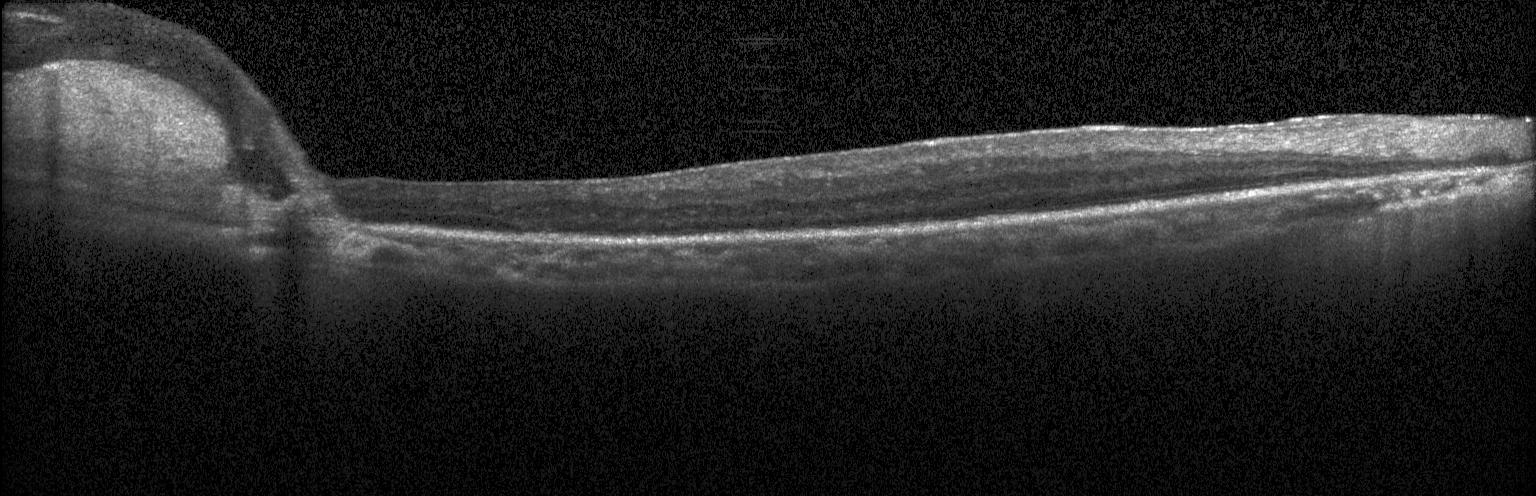
OCT B-scan · through the macula · spectral-domain OCT
Diagnosis: a choroidal neovascular membrane.